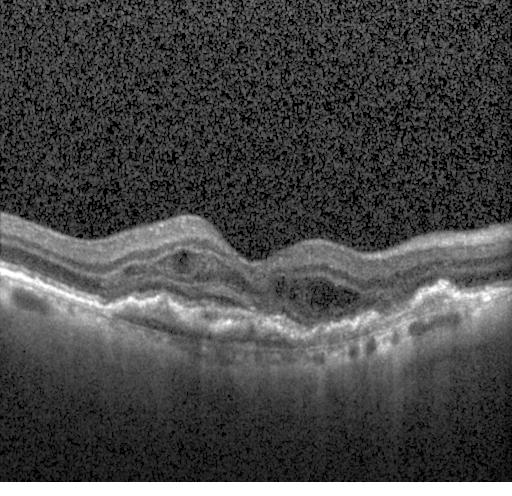 Retinal OCT cross-section.
Finding: a choroidal neovascular membrane.